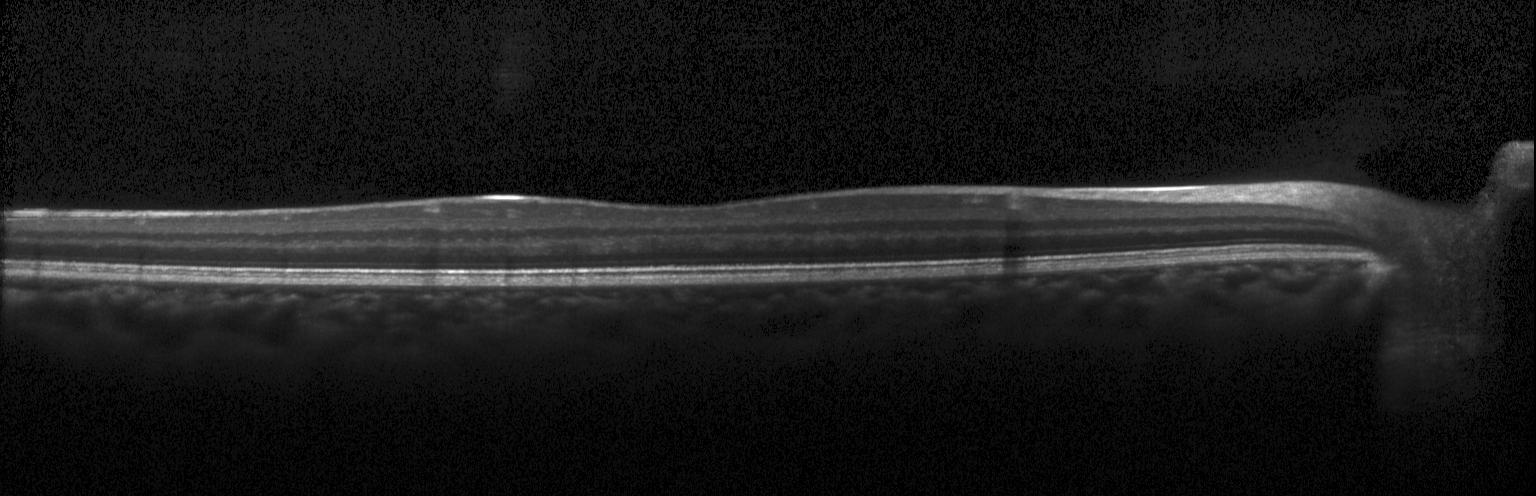
Diagnosis: neither CNV, DME, nor drusen.